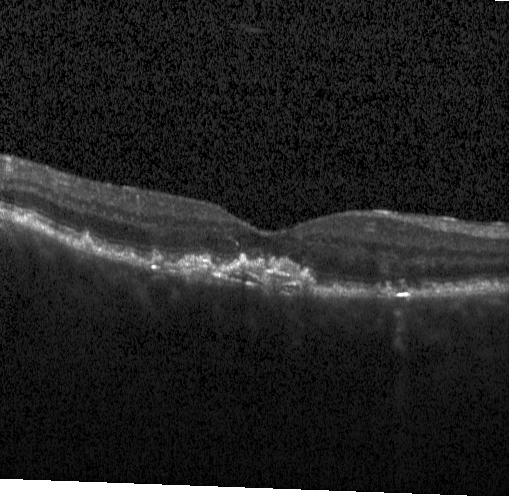

Optical coherence tomography B-scan.
A choroidal neovascular membrane.